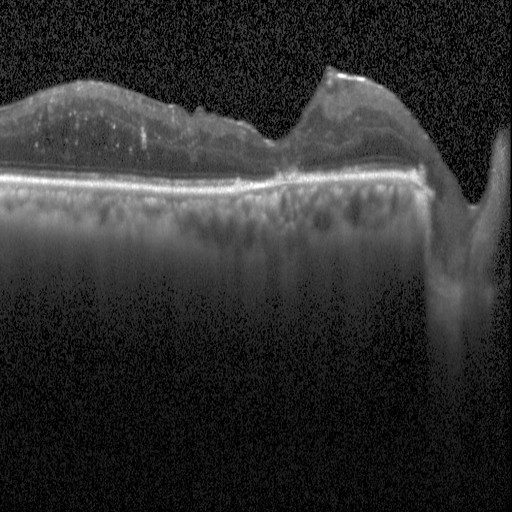
Retinal OCT B-scan. Spectral-domain OCT
Diagnosis: DME.